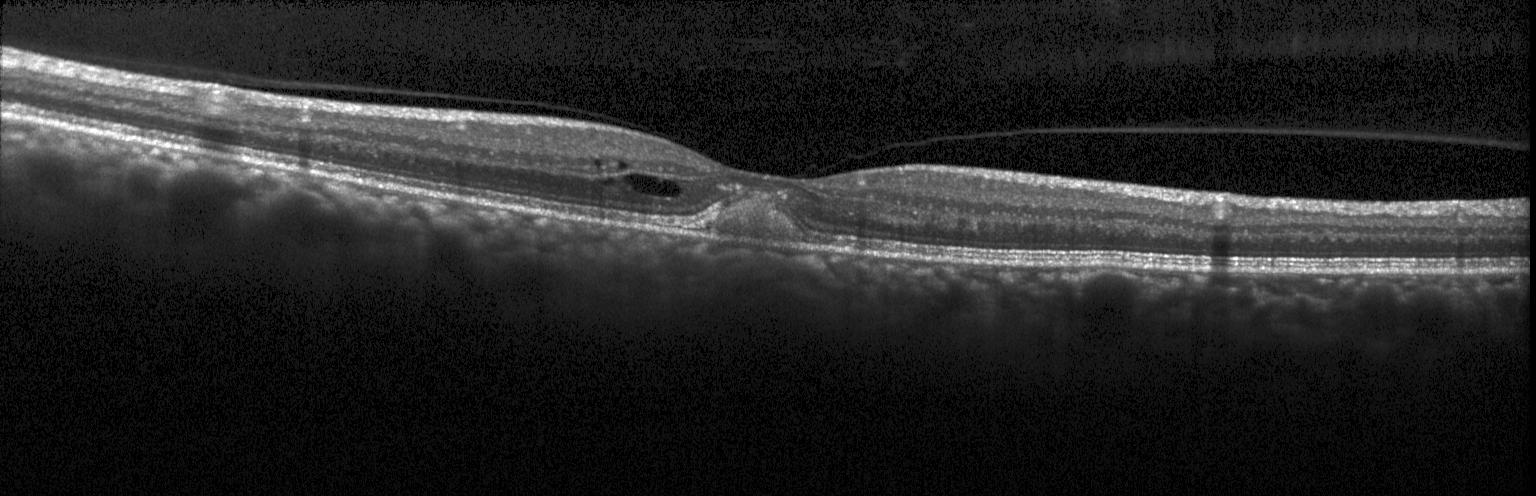
OCT B-scan showing choroidal neovascularization (CNV).